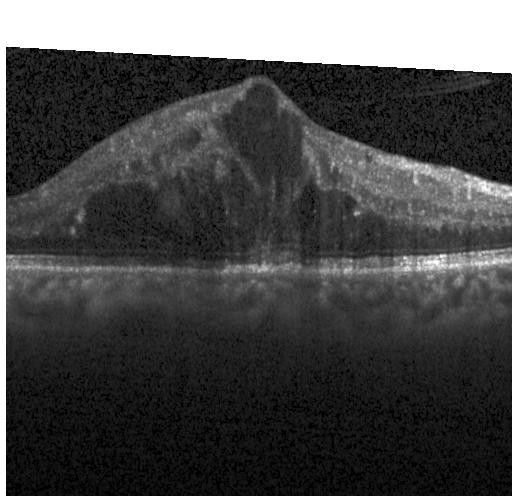

Finding: DME.